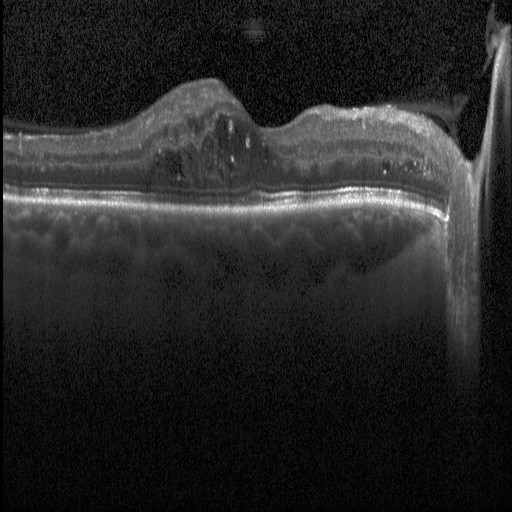

Dx: DME.